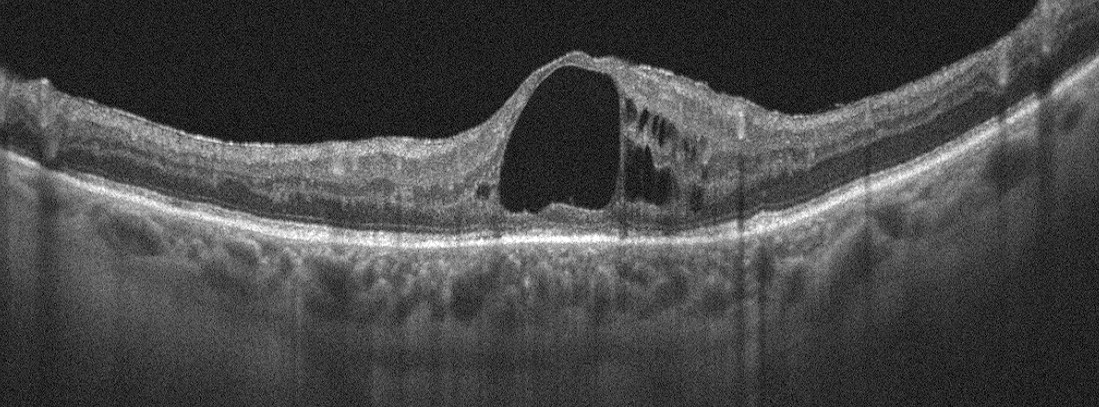
Optovue Avanti RTVue XR, OCT line scan, fovea-centered.
Impression: DME.